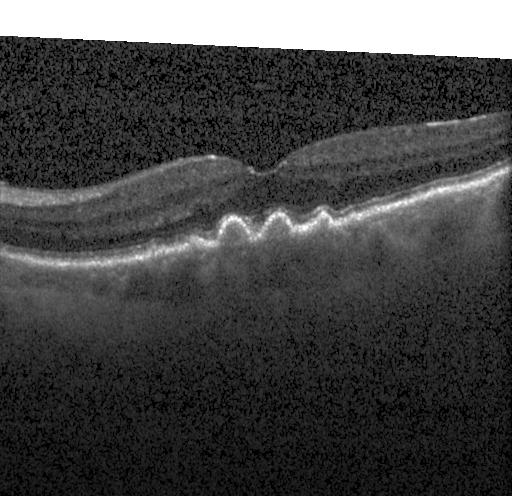 Retinal OCT B-scan
Diagnosis: multiple drusen.